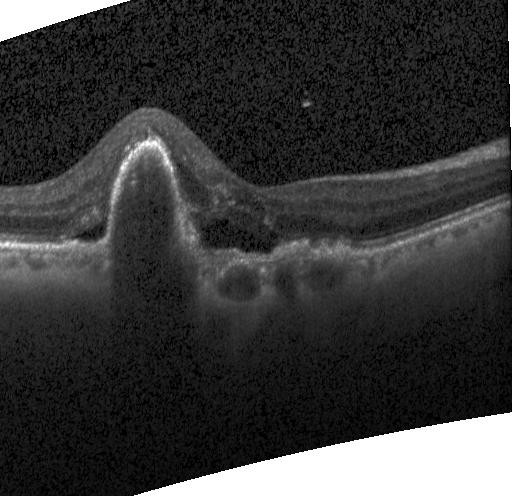
Spectral-domain OCT B-scan: a choroidal neovascular membrane.